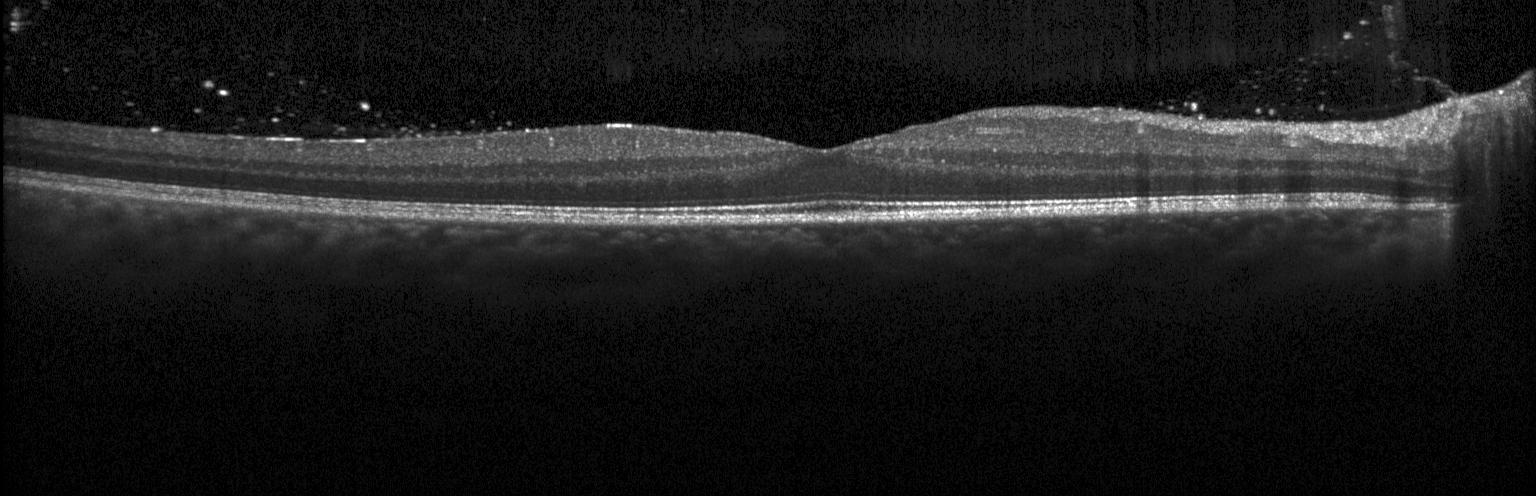

Dx: neither CNV, DME, nor drusen.